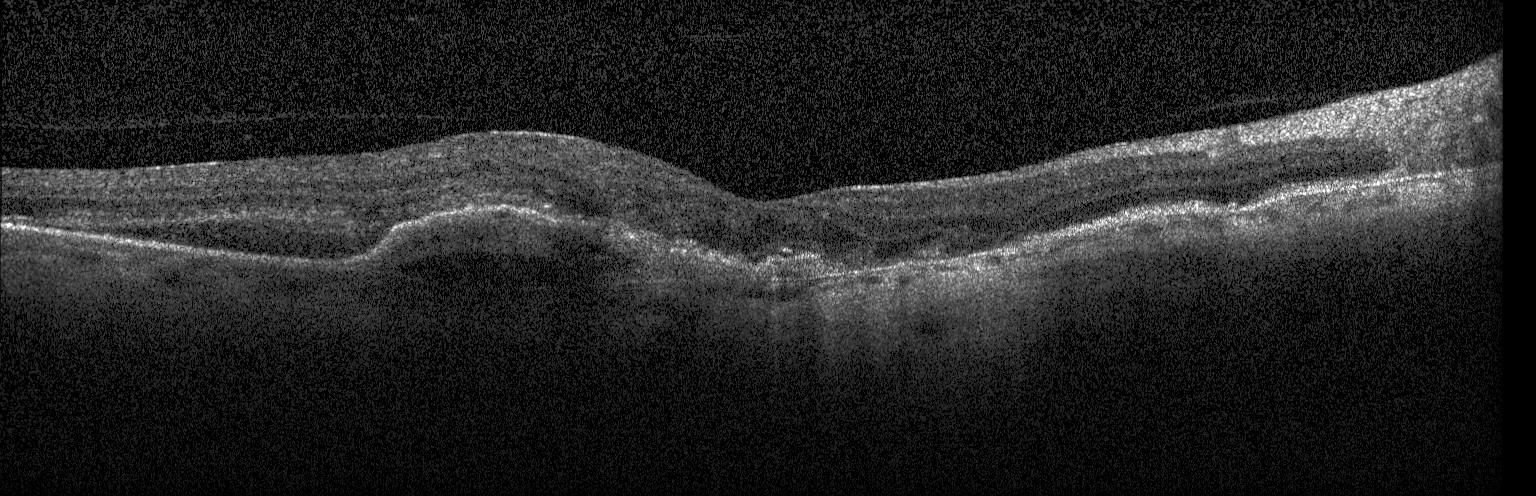
Spectral-domain OCT, OCT B-scan. Impression: CNV.